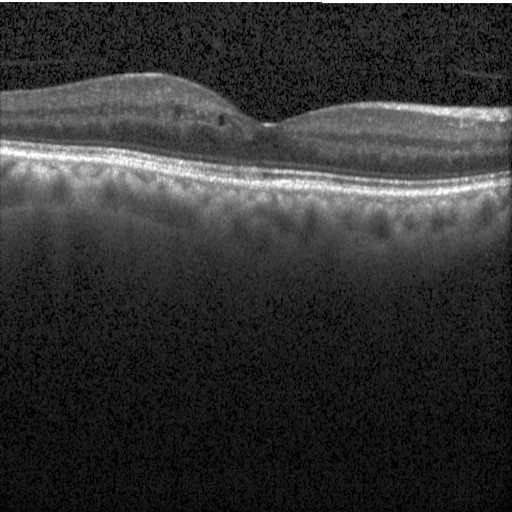
Centered on the fovea; Heidelberg Spectralis; spectral-domain optical coherence tomography; OCT line scan — The scan shows DME.